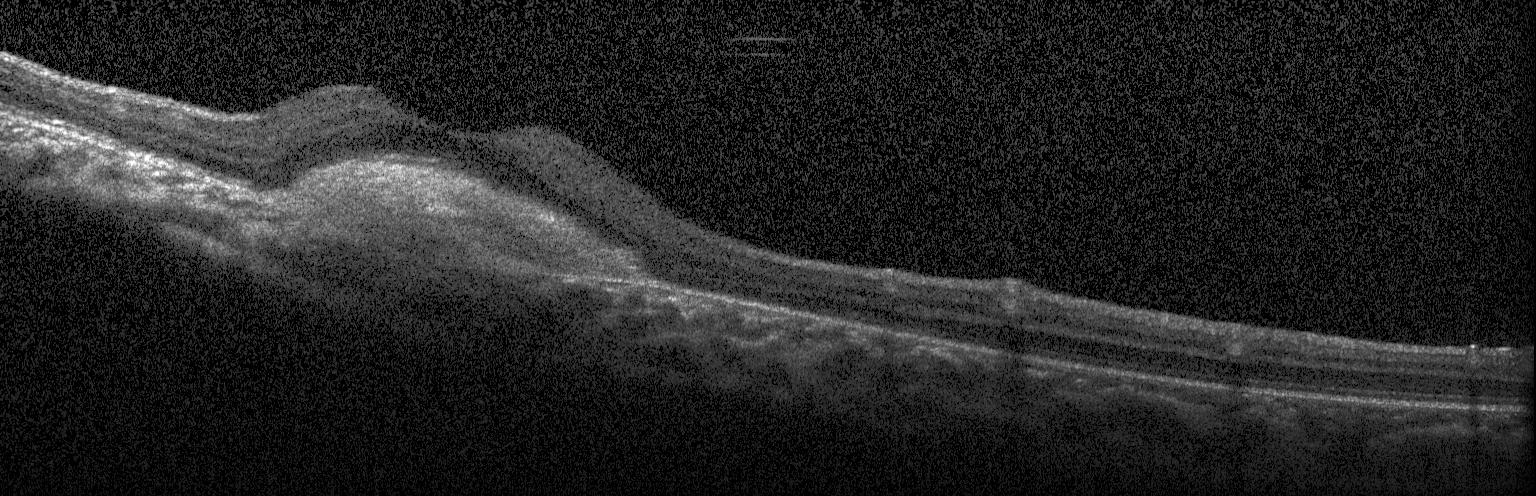

Heidelberg Spectralis OCT system, OCT line scan, spectral-domain optical coherence tomography, through the macula. A choroidal neovascular membrane.